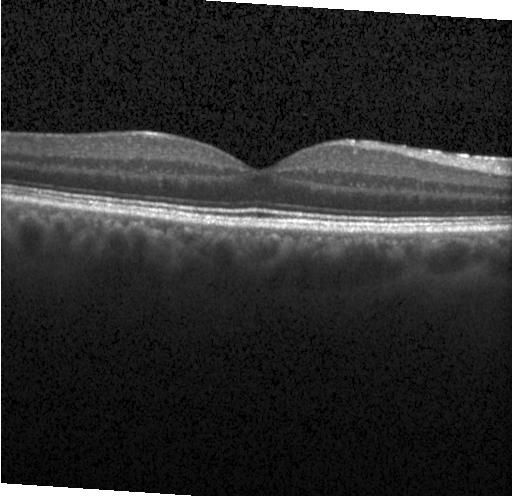 Dx: neither CNV, DME, nor drusen.